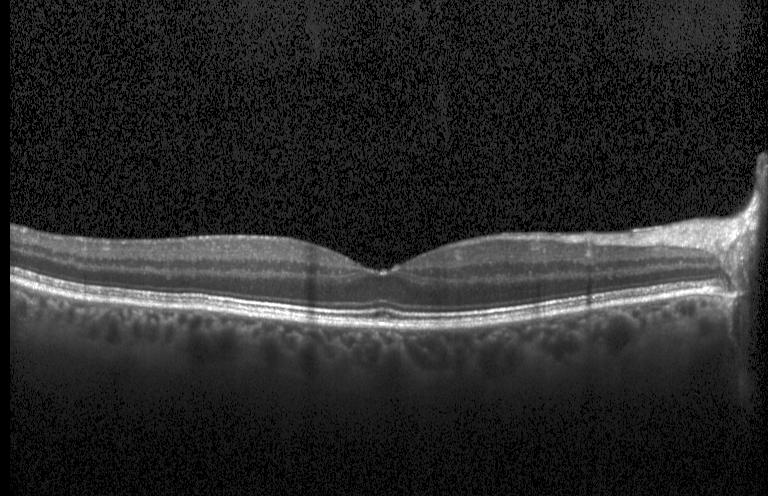
Retinal OCT cross-section. Diagnosis: no CNV, no DME, and no drusen.